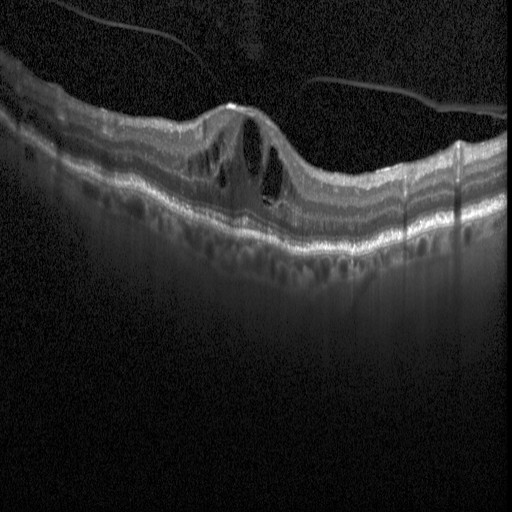 Instrument: Heidelberg Spectralis; spectral-domain OCT; optical coherence tomography scan. Assessment: DME.